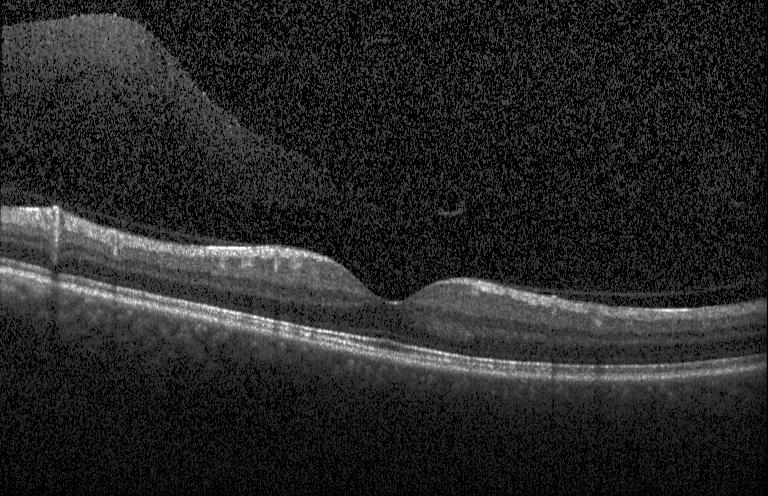 Retinal OCT cross-section — Finding: no CNV, no DME, and no drusen.